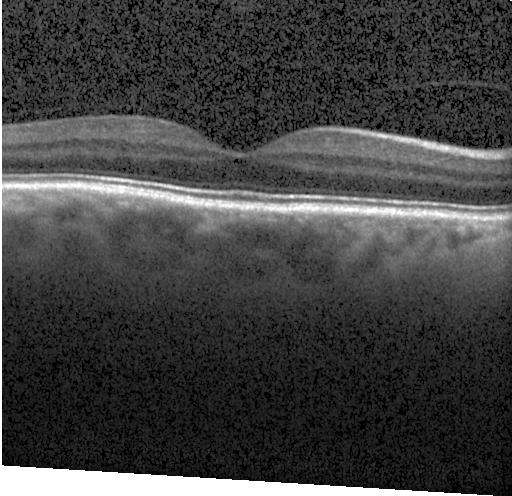 OCT B-scan. Instrument: Heidelberg Spectralis. Spectral-domain OCT. Fovea-centered — No choroidal neovascularization, no diabetic macular edema, and no drusen.